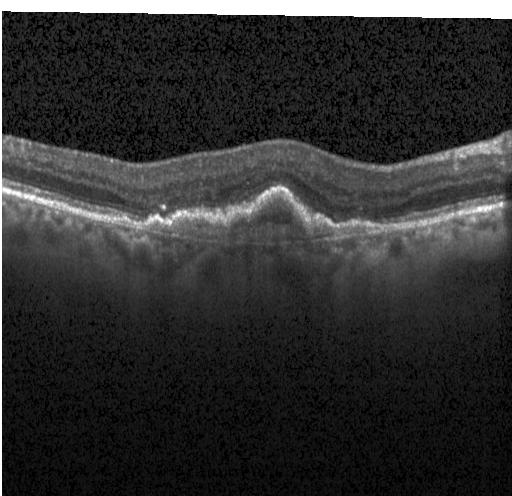
OCT finding: a choroidal neovascular membrane.